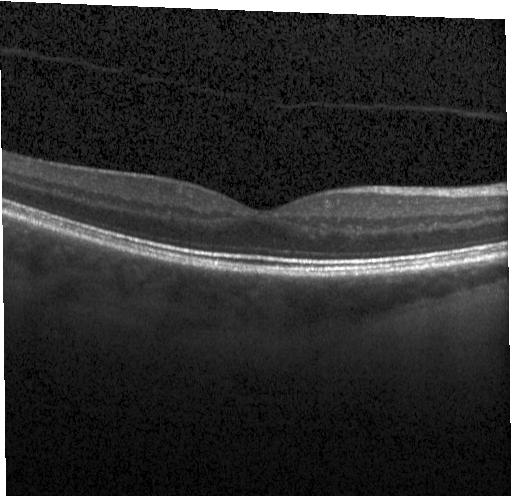 OCT B-scan, acquired on a Heidelberg Spectralis, spectral-domain OCT — Finding: no choroidal neovascularization, diabetic macular edema, or drusen.